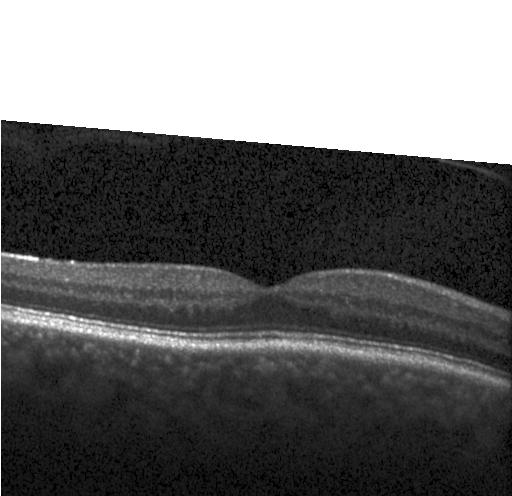
Retinal OCT B-scan; Heidelberg Spectralis OCT system
Finding: no choroidal neovascularization, no diabetic macular edema, and no drusen.